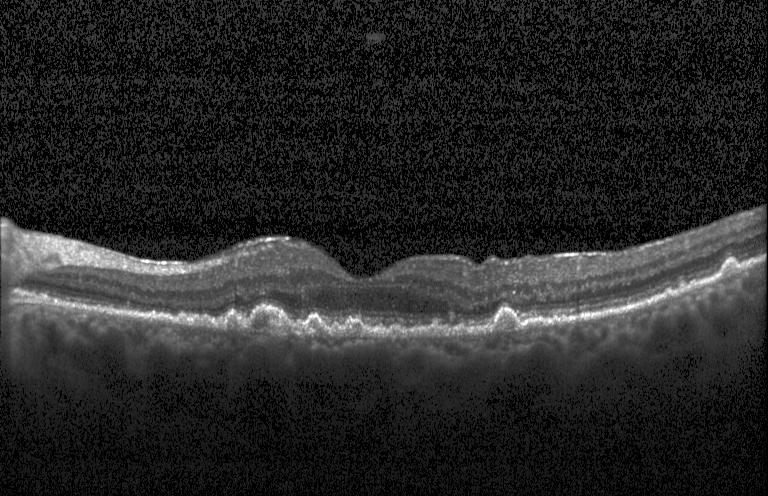
Retinal OCT B-scan — Finding: multiple drusen.